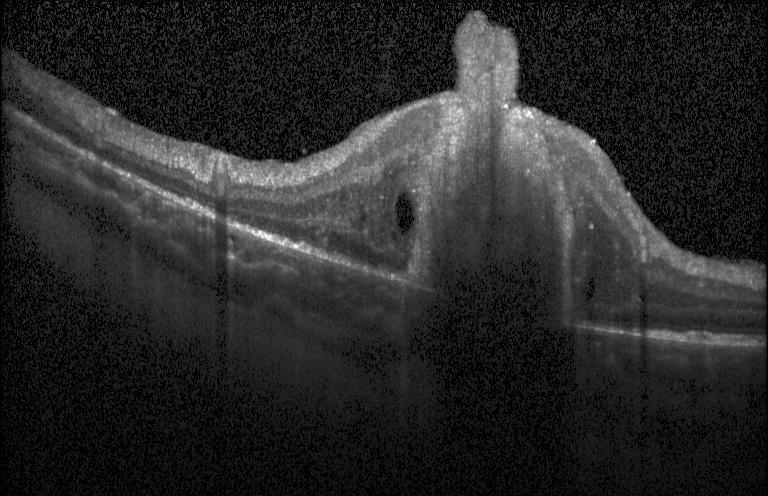

Assessment: a choroidal neovascular membrane.